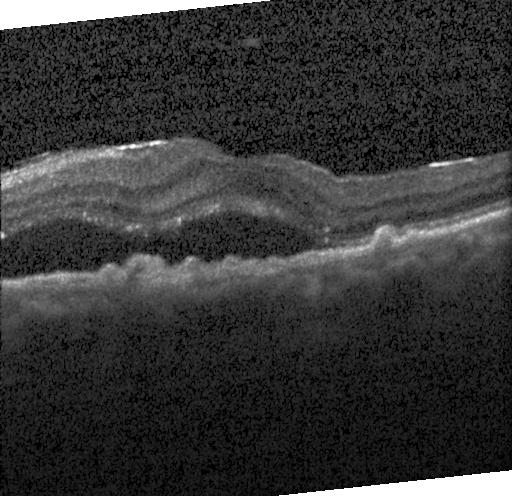 Retinal OCT cross-section; Heidelberg Spectralis OCT system; spectral-domain OCT; fovea-centered
Finding: a choroidal neovascular membrane.